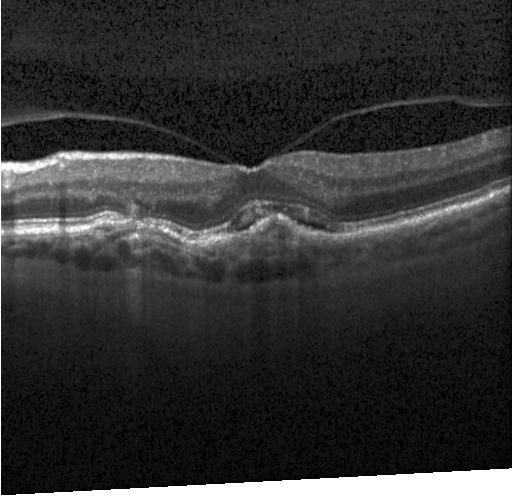

Macular OCT: choroidal neovascularization (CNV).